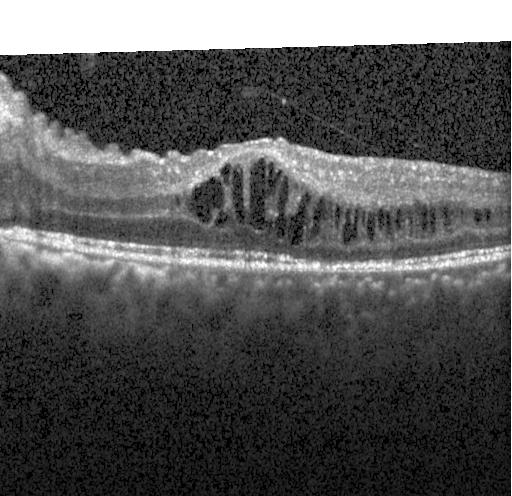

Spectral-domain OCT, instrument: Heidelberg Spectralis, macular scan, optical coherence tomography B-scan — This B-scan demonstrates diabetic macular edema (DME).